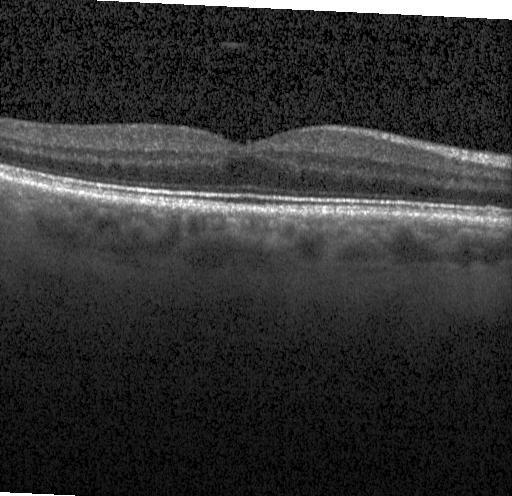 Macular OCT demonstrating neither CNV, DME, nor drusen.